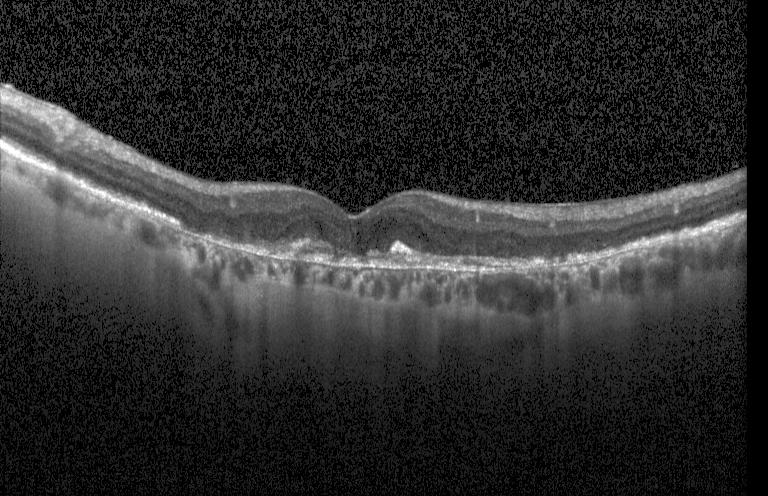

Fovea-centered, Heidelberg Spectralis, OCT B-scan, SD-OCT
Impression: CNV.